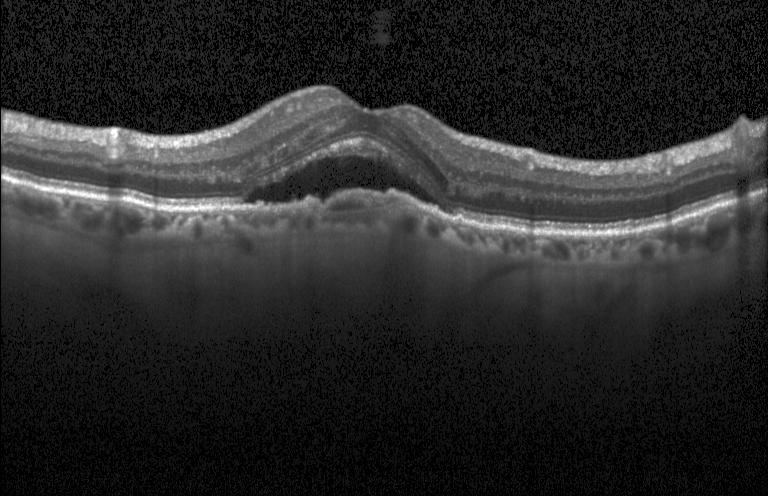

Heidelberg Spectralis OCT system; spectral-domain OCT; optical coherence tomography B-scan
Impression: a choroidal neovascular membrane.